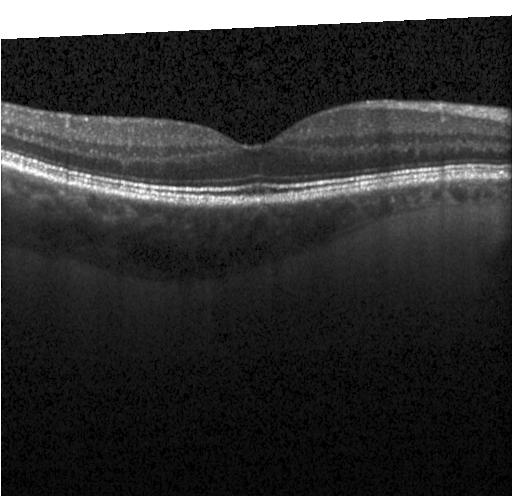

Macular OCT: neither choroidal neovascularization, diabetic macular edema, nor drusen.